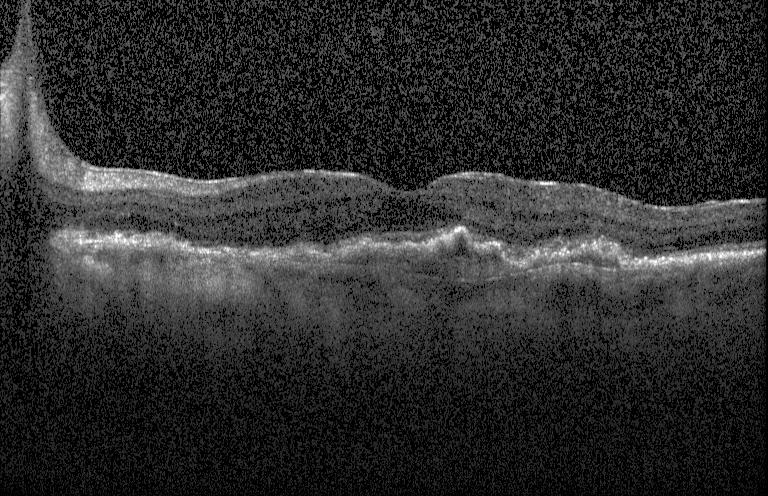 Optical coherence tomography scan; macular scan; SD-OCT; acquired on a Heidelberg Spectralis.
Finding: choroidal neovascularization.